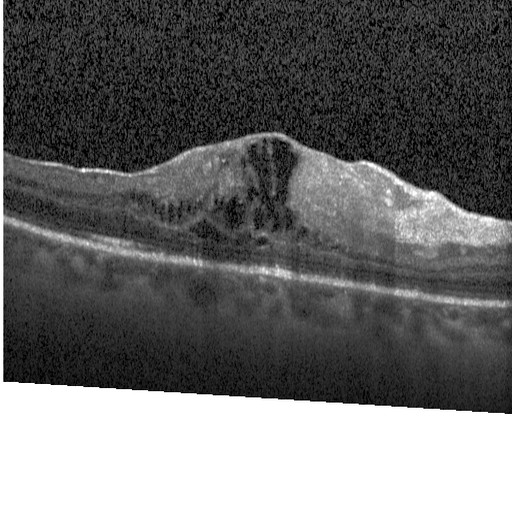
Impression: diabetic macular edema.